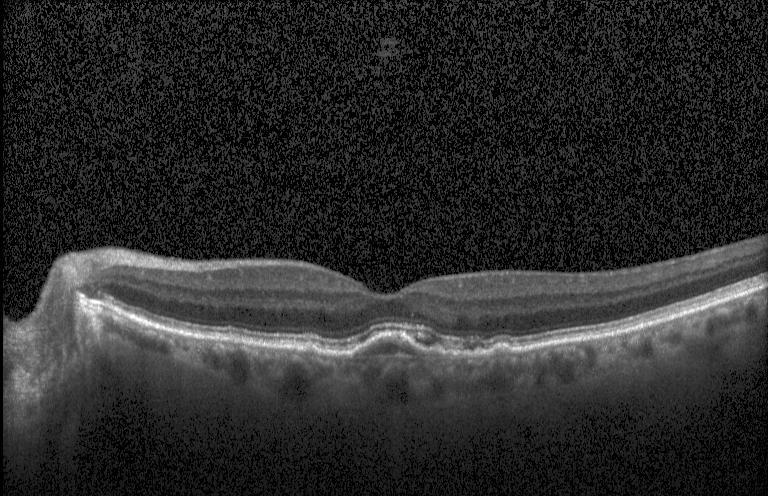
Macular scan. Spectral-domain optical coherence tomography. OCT line scan — The scan shows choroidal neovascularization.